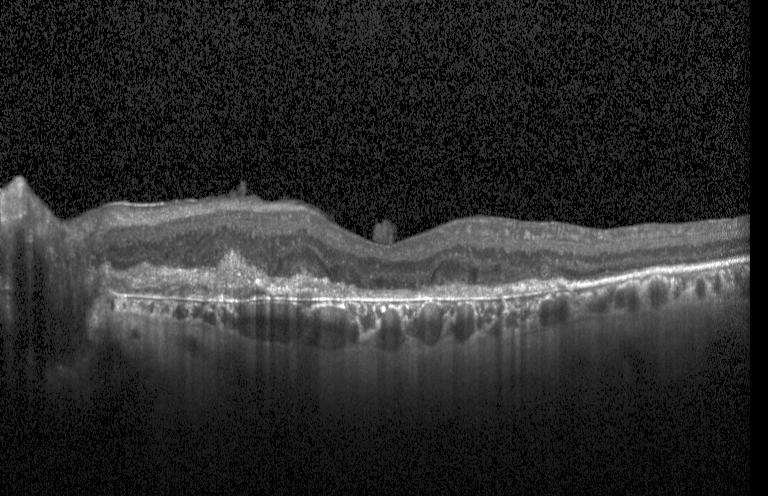 Optical coherence tomography scan. Diagnosis: choroidal neovascularization.